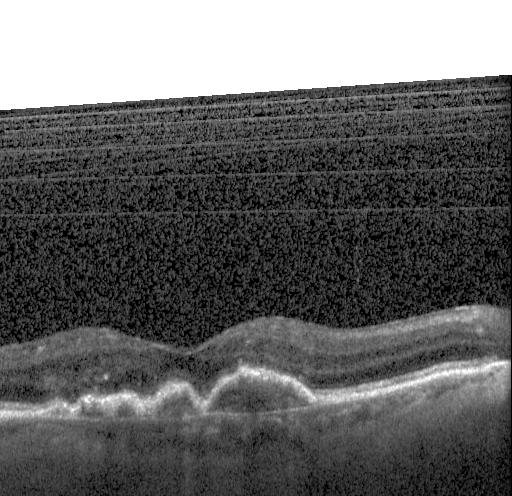

Retinal OCT cross-section · Heidelberg Spectralis · through the macula.
Finding: a choroidal neovascular membrane.